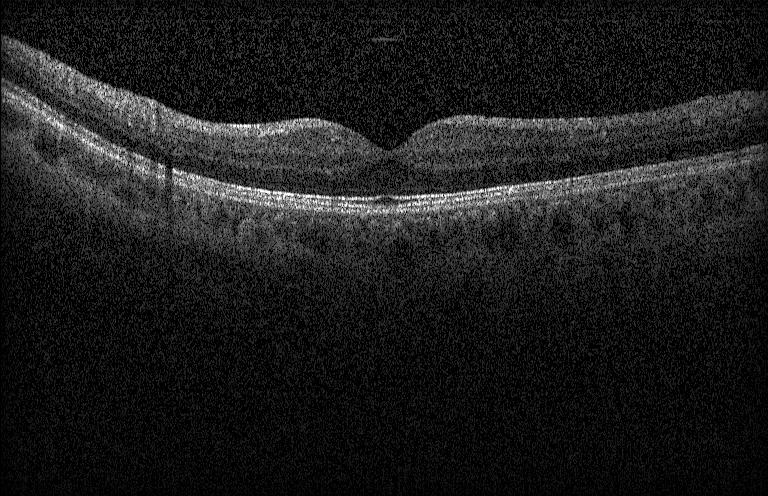 OCT scan showing no evidence of choroidal neovascularization, diabetic macular edema, or drusen.